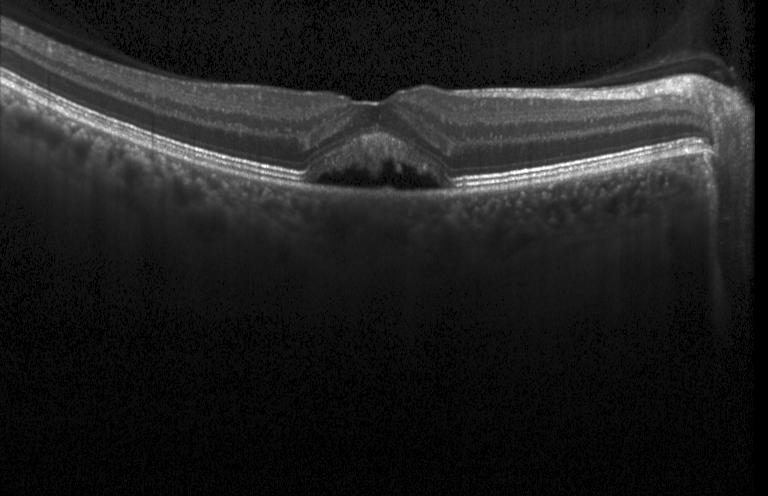
Finding: a choroidal neovascular membrane.